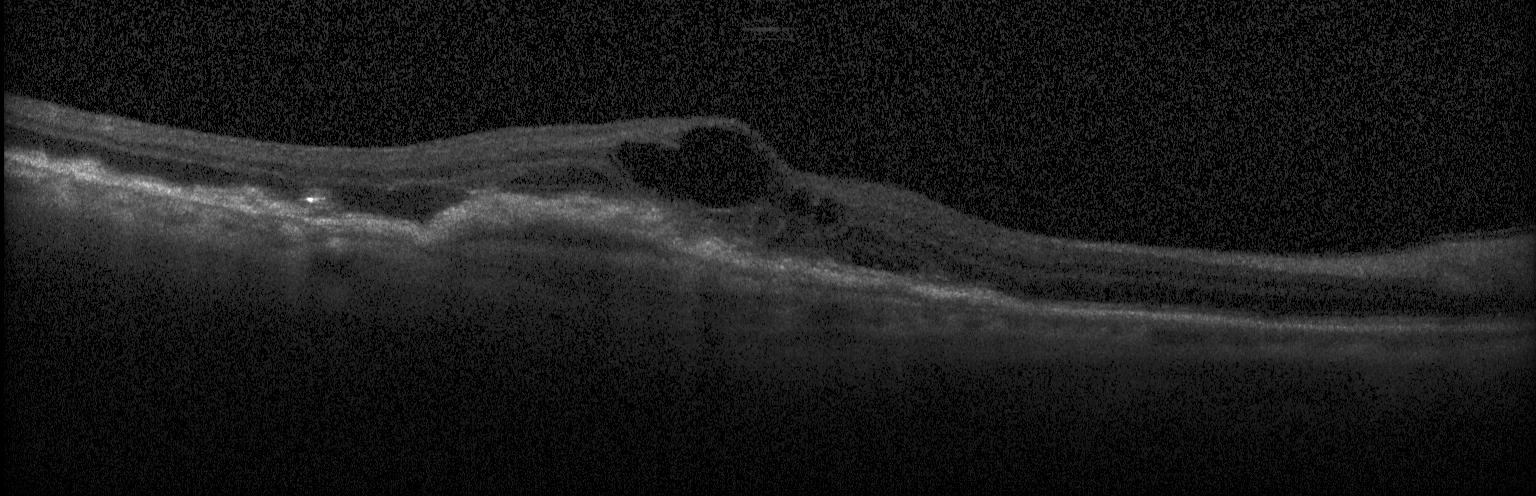
Macular OCT demonstrating a choroidal neovascular membrane.